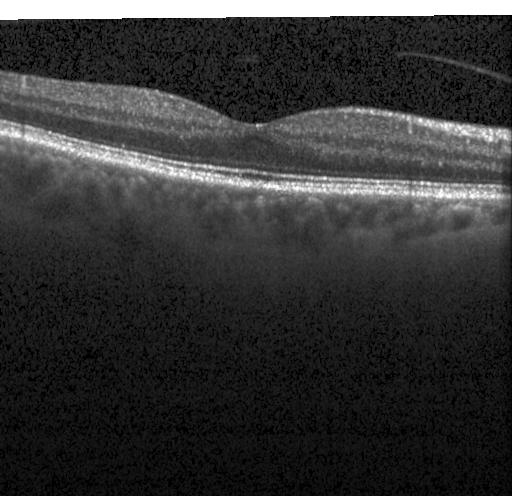
Retinal OCT B-scan. Diagnosis: neither choroidal neovascularization, diabetic macular edema, nor drusen.